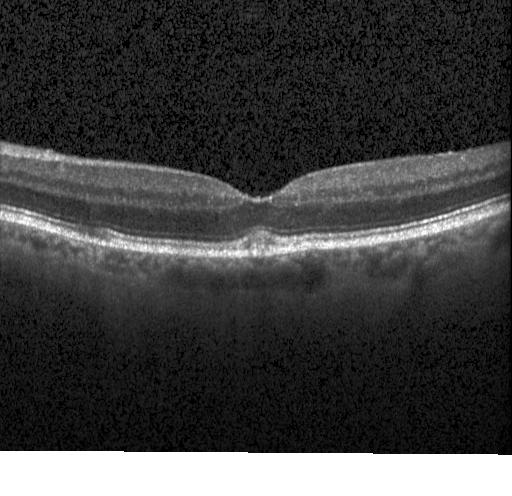 OCT B-scan, through the macula. Finding: sub-RPE drusenoid deposits.